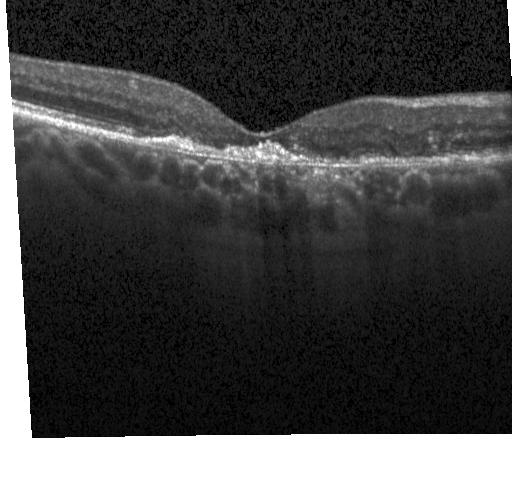

Heidelberg Spectralis; horizontal scan through the fovea; OCT B-scan; spectral-domain optical coherence tomography.
Assessment: a choroidal neovascular membrane.